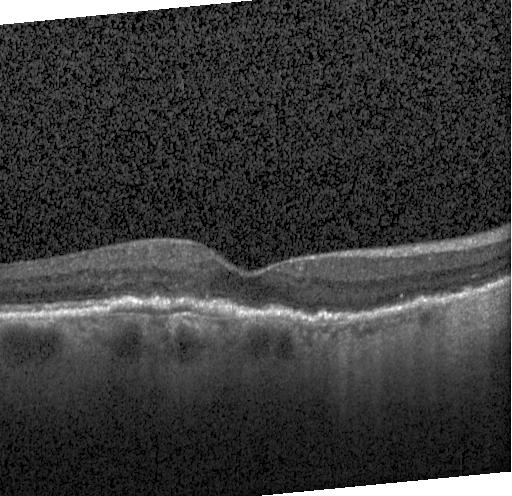

SD-OCT · acquired on a Heidelberg Spectralis · OCT B-scan — Impression: a choroidal neovascular membrane.